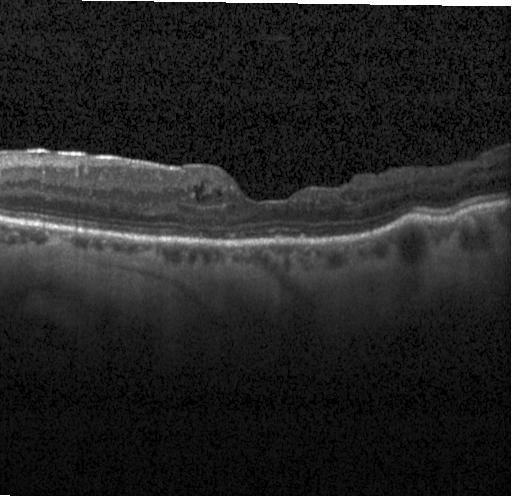

Spectral-domain optical coherence tomography. Through the macula. Heidelberg Spectralis OCT system. OCT line scan — This B-scan demonstrates diabetic macular edema (DME).